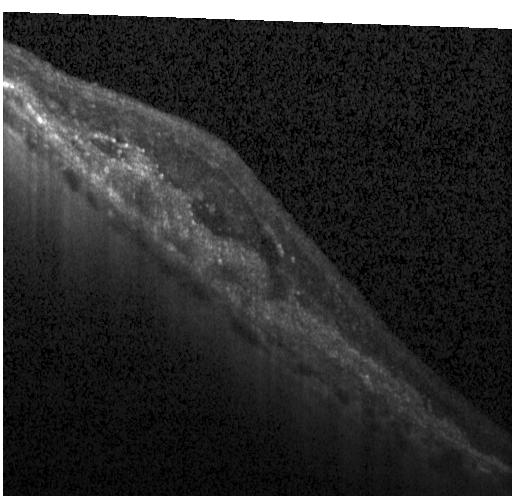 Retinal OCT B-scan · spectral-domain OCT.
This B-scan demonstrates a choroidal neovascular membrane.